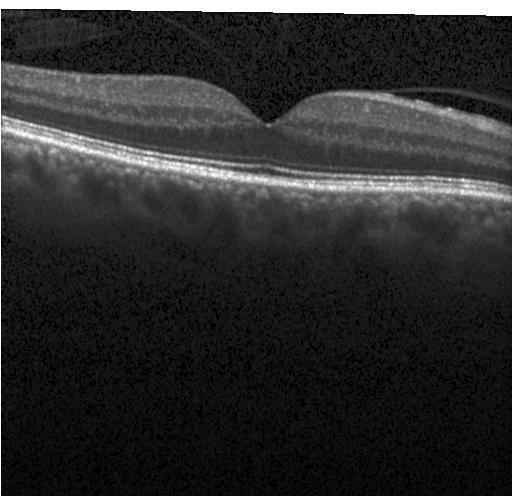

Macular scan. Retinal OCT B-scan
No choroidal neovascularization, diabetic macular edema, or drusen.